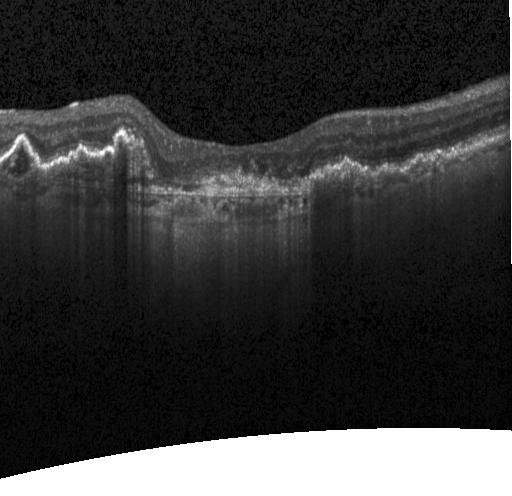

Finding: choroidal neovascularization.